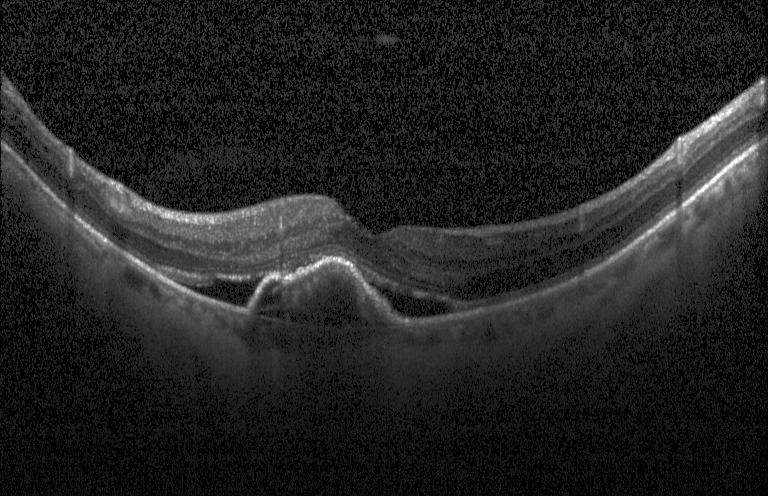
This B-scan demonstrates a choroidal neovascular membrane.